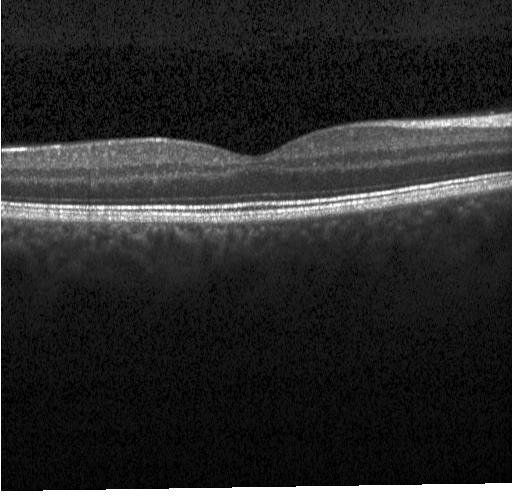

No choroidal neovascularization, no diabetic macular edema, and no drusen.